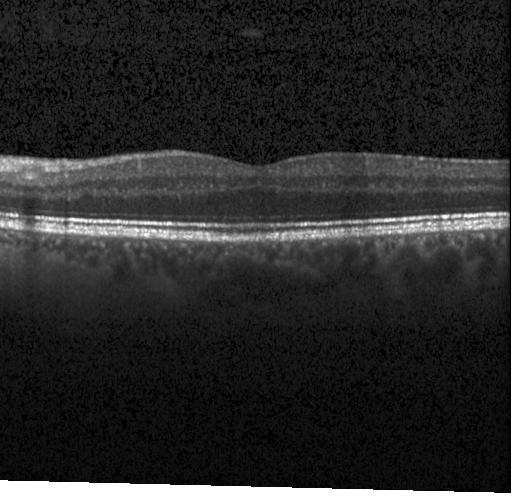
Macular scan. Heidelberg Spectralis OCT system. Optical coherence tomography scan.
Impression: neither choroidal neovascularization, diabetic macular edema, nor drusen.